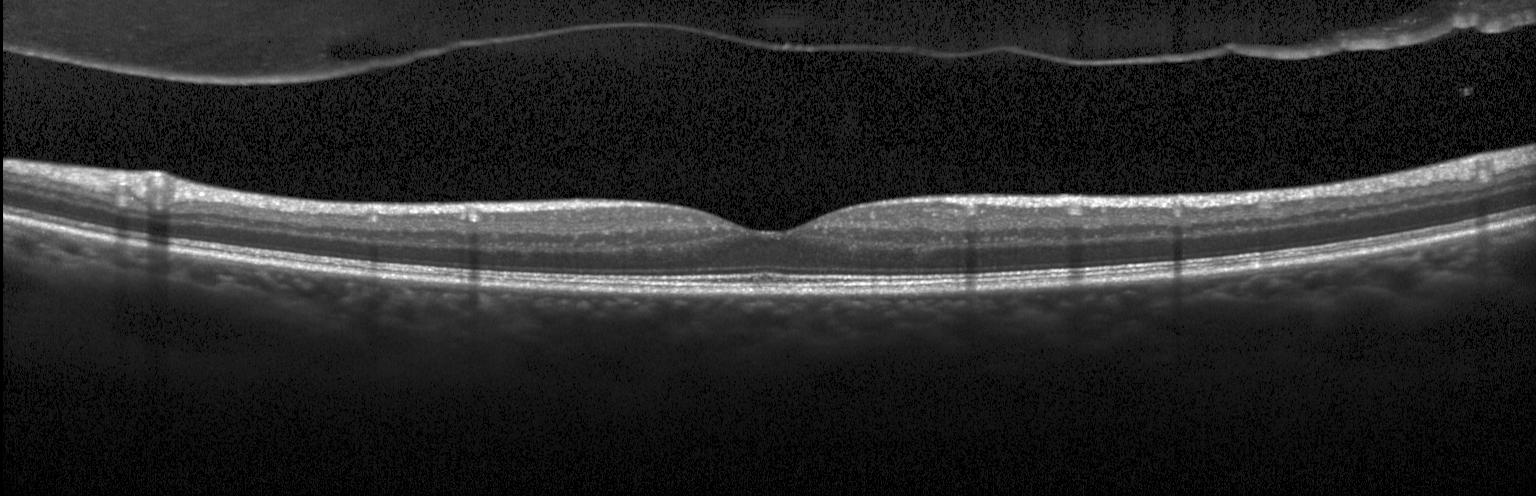 Finding: no choroidal neovascularization, no diabetic macular edema, and no drusen.